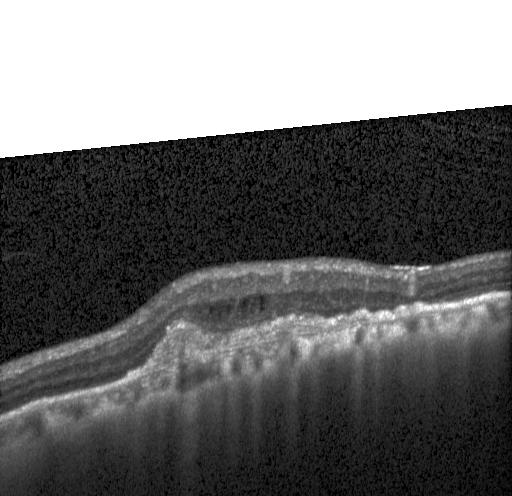
Retinal OCT cross-section; spectral-domain OCT; Heidelberg Spectralis OCT system. Impression: a choroidal neovascular membrane.